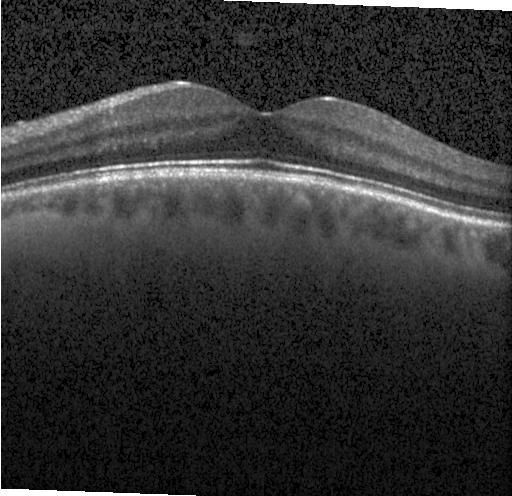 Heidelberg Spectralis OCT system. Macular scan. OCT line scan — Diagnosis: no CNV, DME, or drusen.